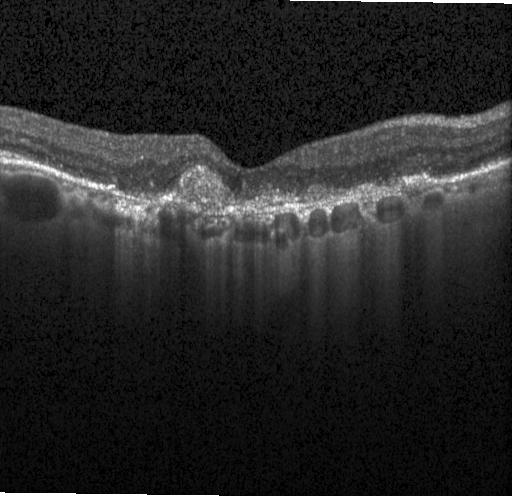
Macular OCT: choroidal neovascularization (CNV).